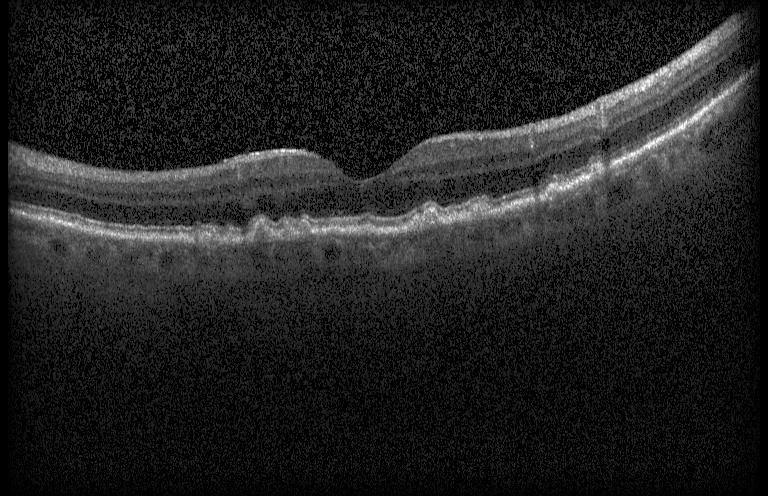 OCT B-scan. Acquired on a Heidelberg Spectralis — OCT finding: sub-RPE drusenoid deposits.